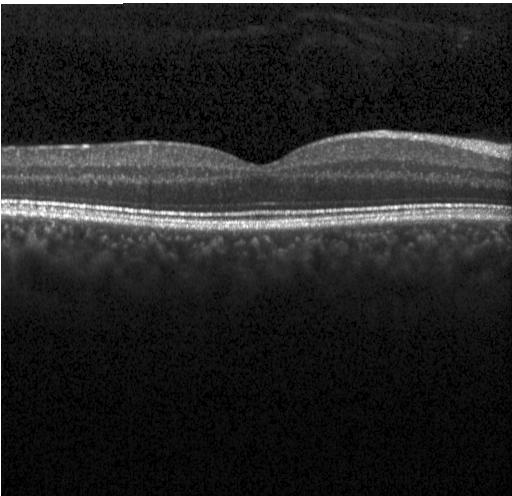 Optical coherence tomography scan; spectral-domain optical coherence tomography.
The scan shows no evidence of choroidal neovascularization, diabetic macular edema, or drusen.